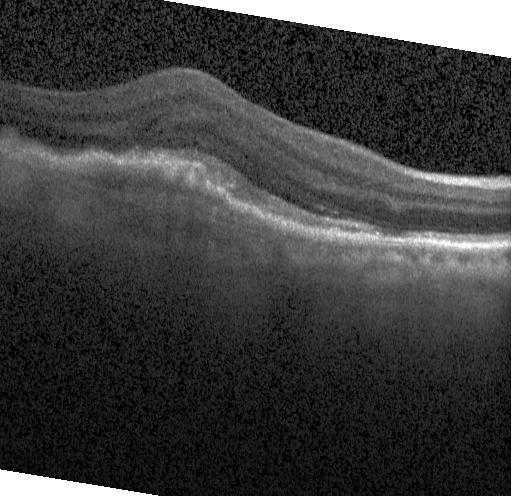
Optical coherence tomography B-scan.
The scan shows a choroidal neovascular membrane.